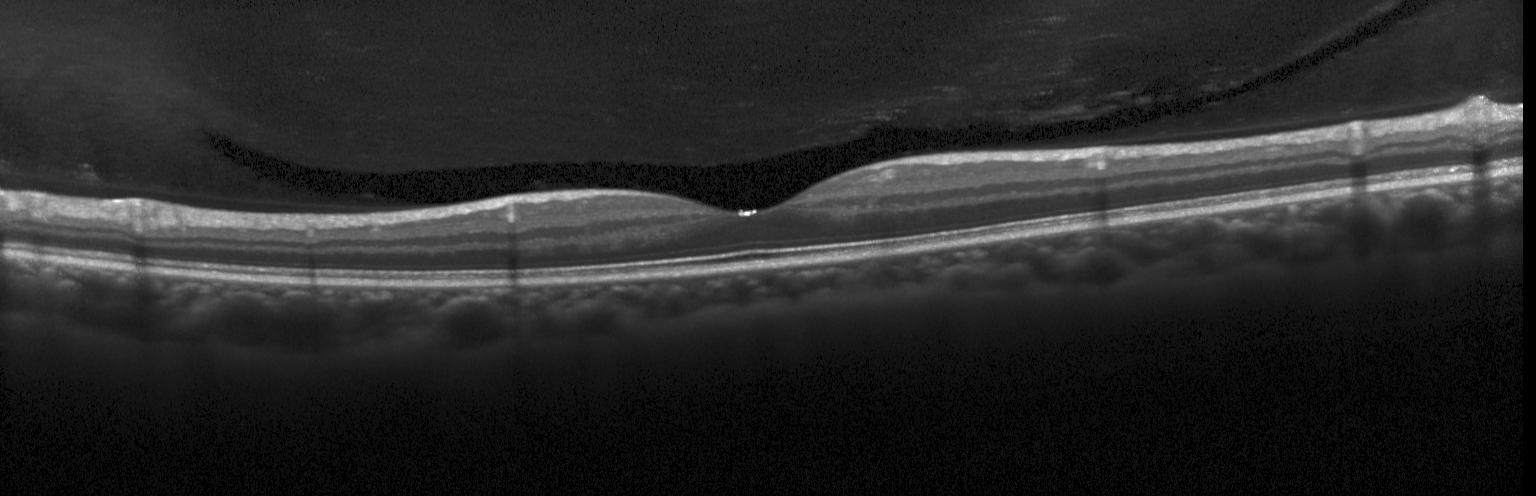

Spectral-domain OCT; optical coherence tomography B-scan — Macular OCT: neither choroidal neovascularization, diabetic macular edema, nor drusen.